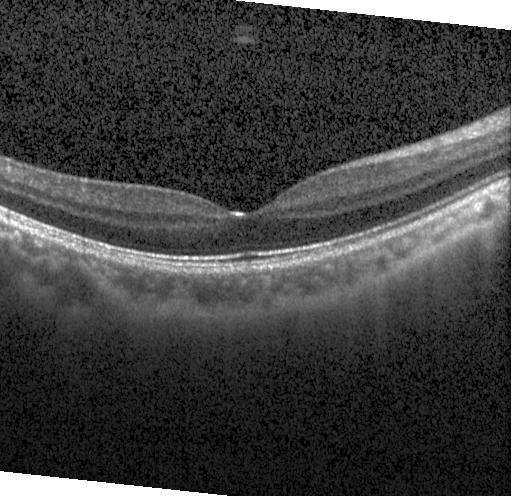 OCT finding: no evidence of choroidal neovascularization, diabetic macular edema, or drusen.